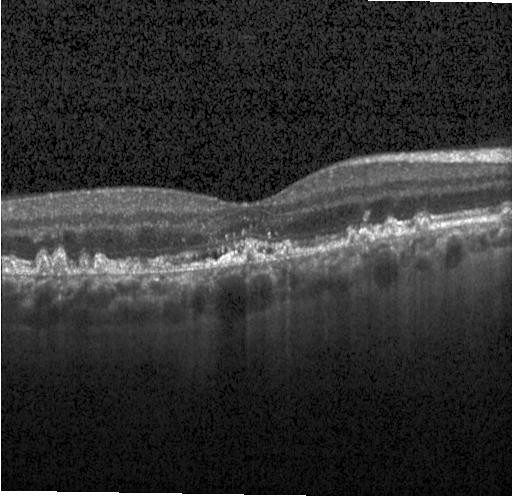

Assessment: a choroidal neovascular membrane.